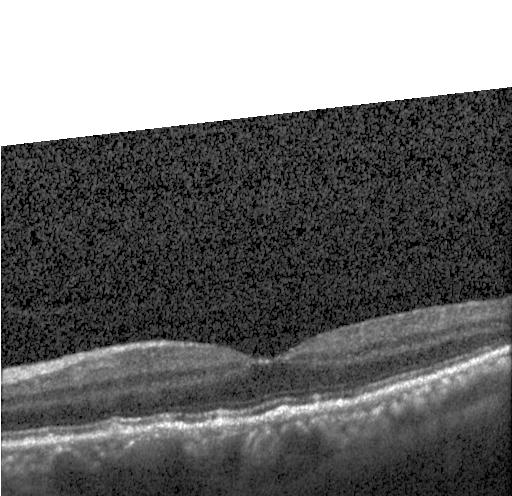 Retinal OCT B-scan — Finding: multiple drusen.